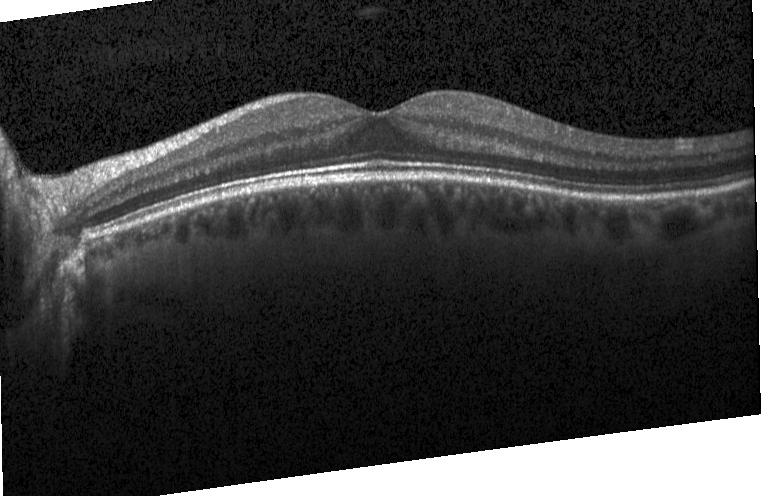
Spectral-domain optical coherence tomography. Retinal OCT cross-section — No choroidal neovascularization, no diabetic macular edema, and no drusen.